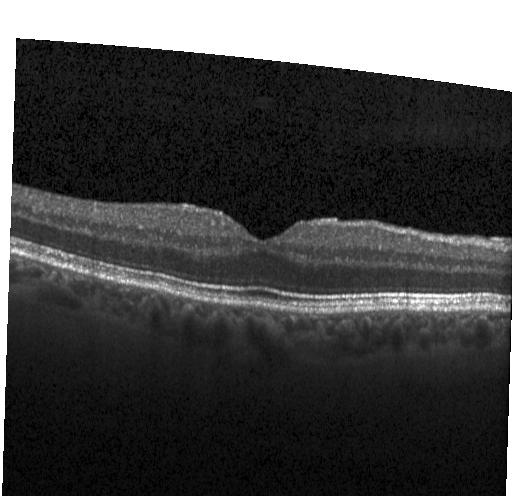
OCT B-scan.
This B-scan demonstrates no choroidal neovascularization, diabetic macular edema, or drusen.